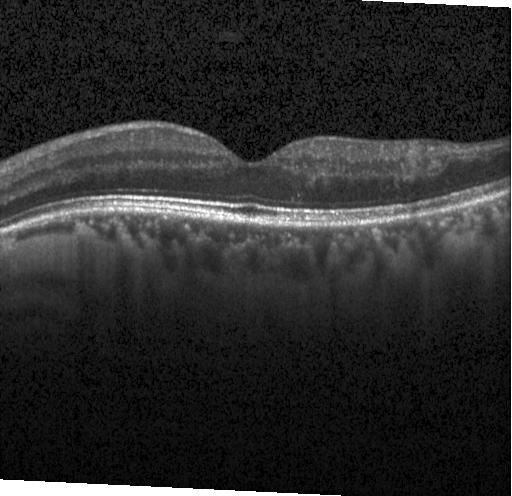 Retinal OCT B-scan · horizontal scan through the fovea · spectral-domain OCT
No choroidal neovascularization, no diabetic macular edema, and no drusen.